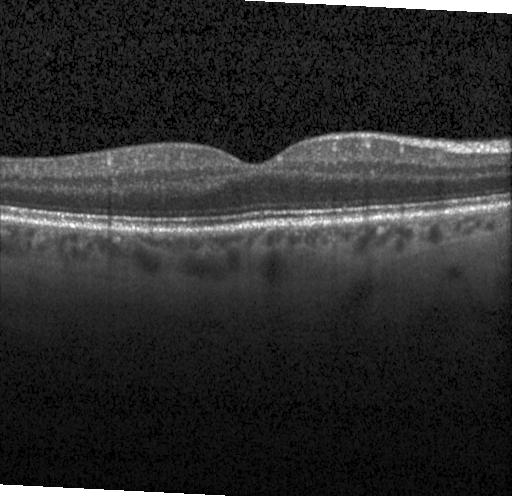

Finding: no choroidal neovascularization, no diabetic macular edema, and no drusen.